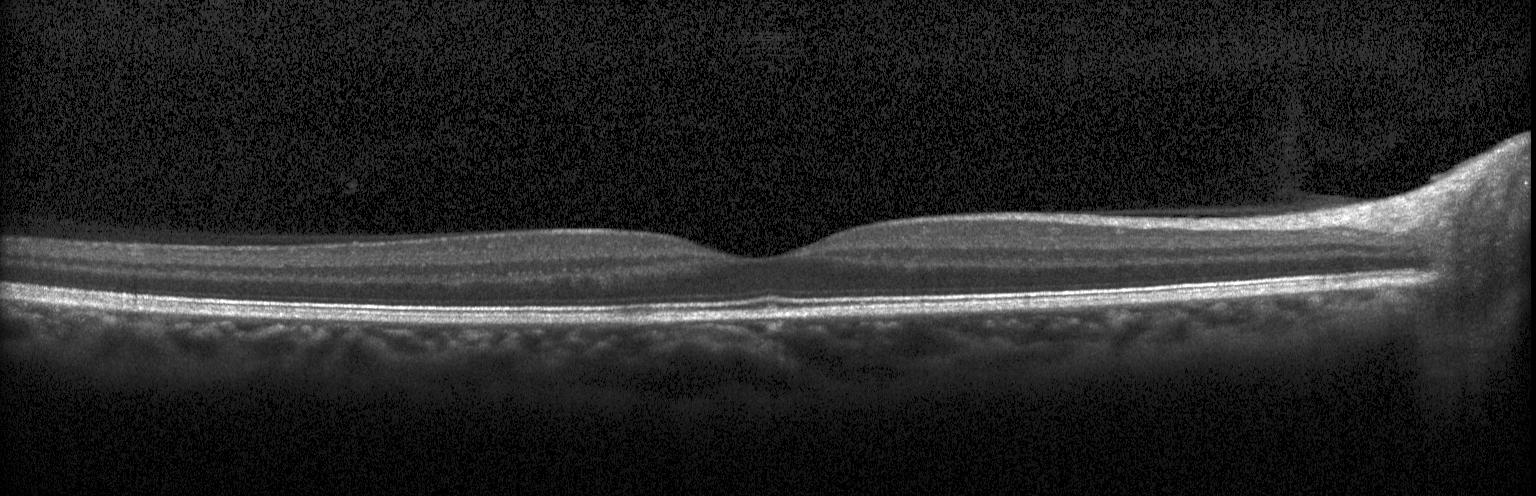

Optical coherence tomography scan, horizontal scan through the fovea — Finding: no evidence of CNV, DME, or drusen.